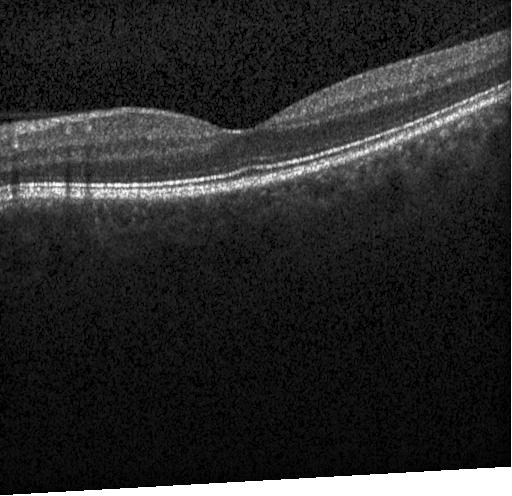
Acquired on a Heidelberg Spectralis · retinal OCT B-scan — Impression: no evidence of choroidal neovascularization, diabetic macular edema, or drusen.